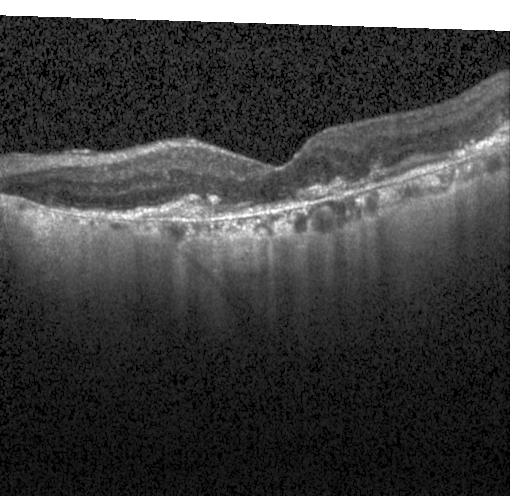

Spectral-domain OCT, macular scan, OCT line scan. This B-scan demonstrates a choroidal neovascular membrane.